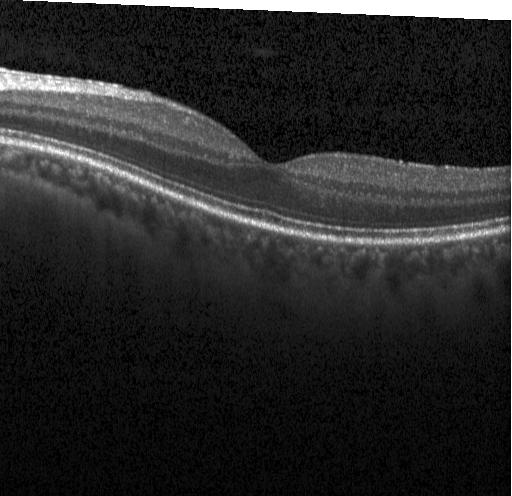
OCT scan showing neither choroidal neovascularization, diabetic macular edema, nor drusen.